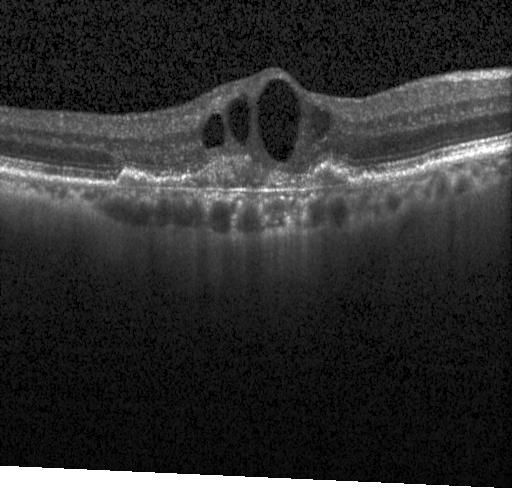

Heidelberg Spectralis OCT system, centered on the fovea, spectral-domain optical coherence tomography, optical coherence tomography B-scan
Impression: CNV.